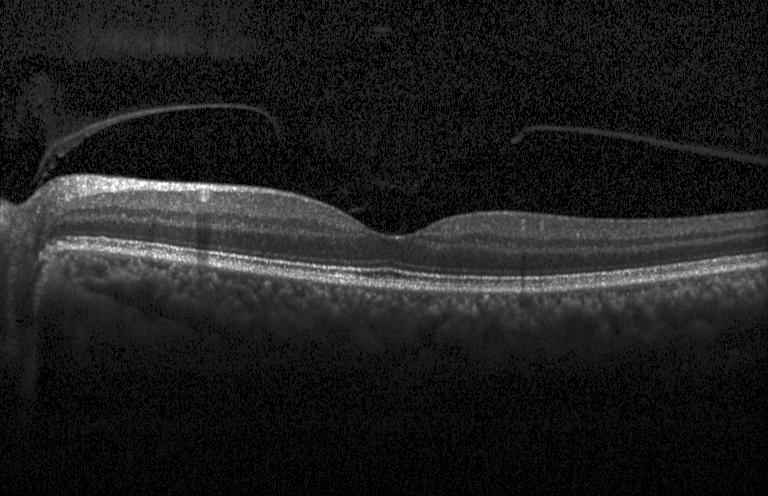 Horizontal scan through the fovea, retinal OCT B-scan. Dx: neither choroidal neovascularization, diabetic macular edema, nor drusen.